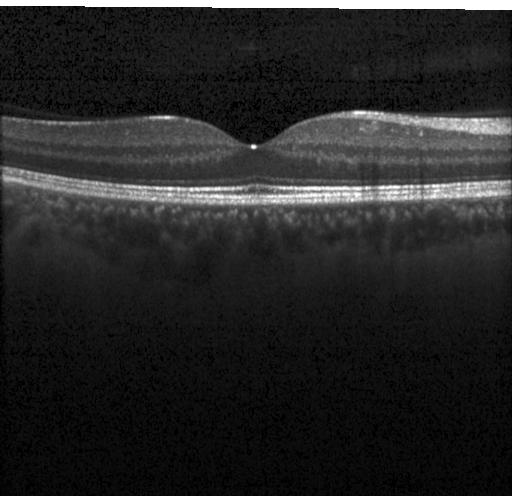
Acquired on a Heidelberg Spectralis · OCT line scan · SD-OCT.
Finding: no CNV, DME, or drusen.